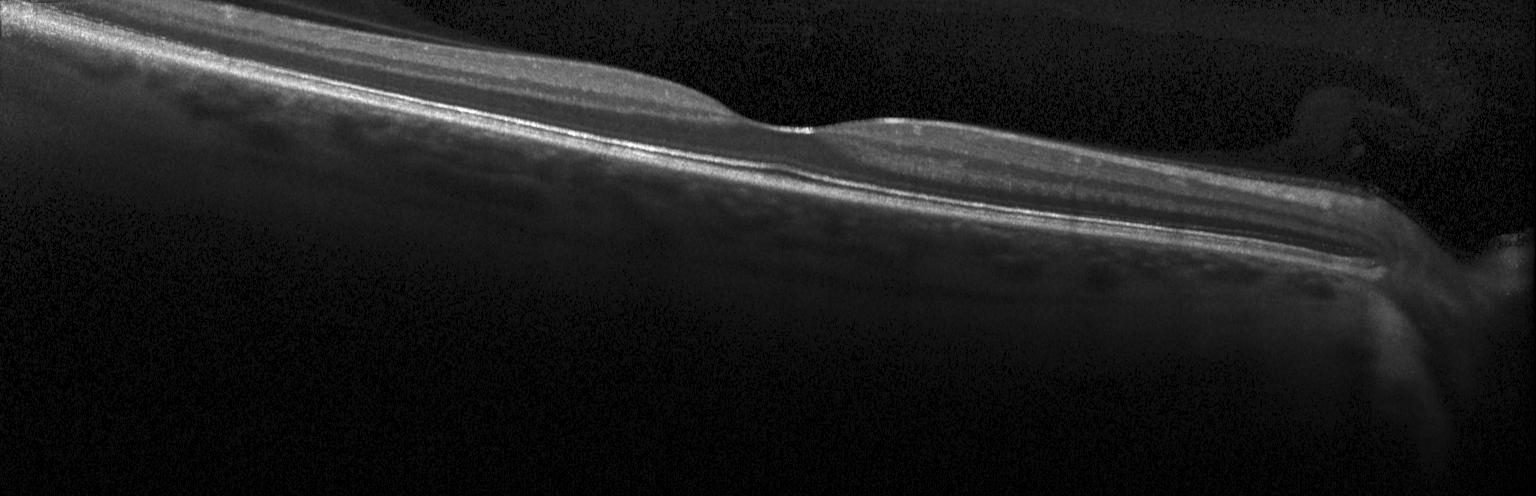
Macular scan; SD-OCT; acquired on a Heidelberg Spectralis; OCT B-scan — Neither choroidal neovascularization, diabetic macular edema, nor drusen.